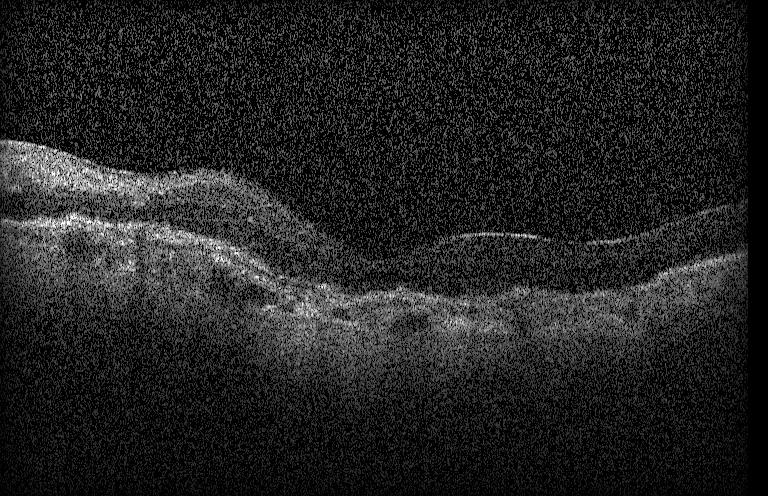

Instrument: Heidelberg Spectralis, retinal OCT cross-section. The scan shows a choroidal neovascular membrane.